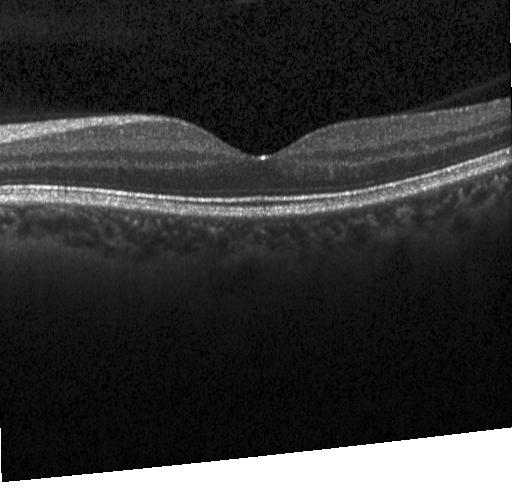

OCT line scan · fovea-centered. Impression: no CNV, no DME, and no drusen.